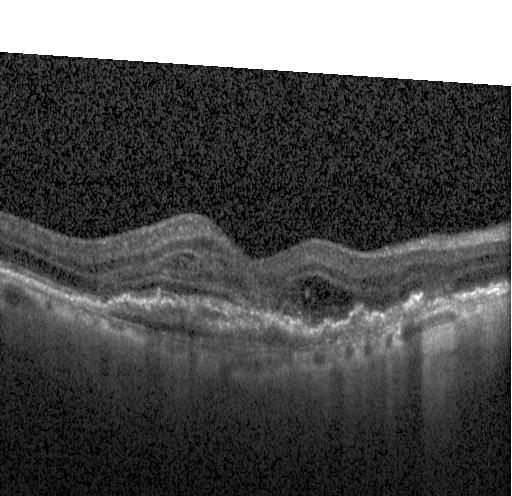 OCT B-scan showing a choroidal neovascular membrane.